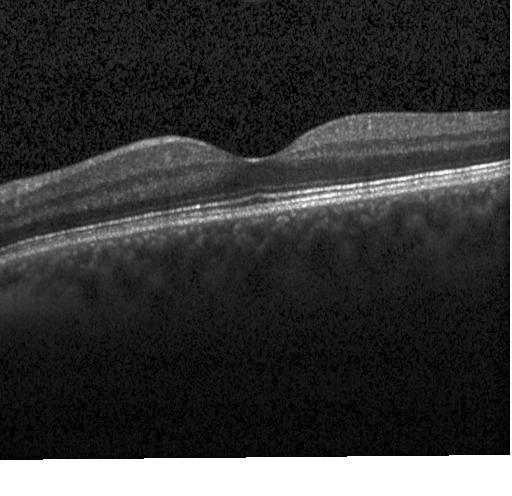
Optical coherence tomography scan · spectral-domain optical coherence tomography
Assessment: no choroidal neovascularization, diabetic macular edema, or drusen.